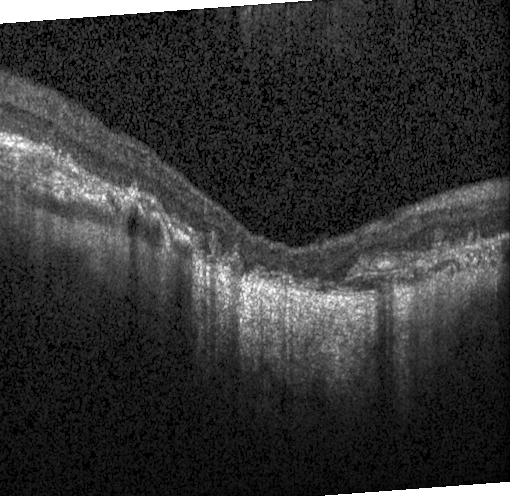 OCT line scan, horizontal scan through the fovea, spectral-domain OCT, Heidelberg Spectralis.
Impression: a choroidal neovascular membrane.